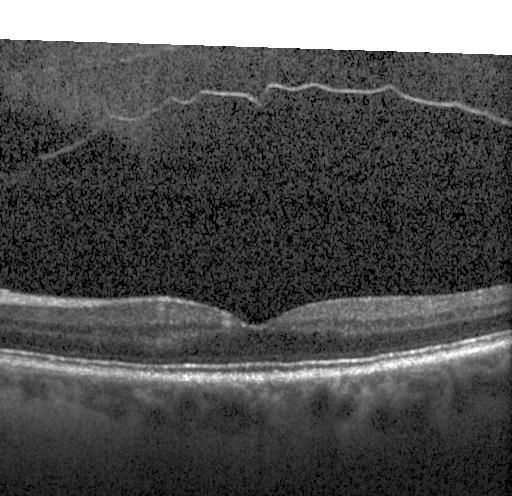

Assessment: no choroidal neovascularization, no diabetic macular edema, and no drusen.